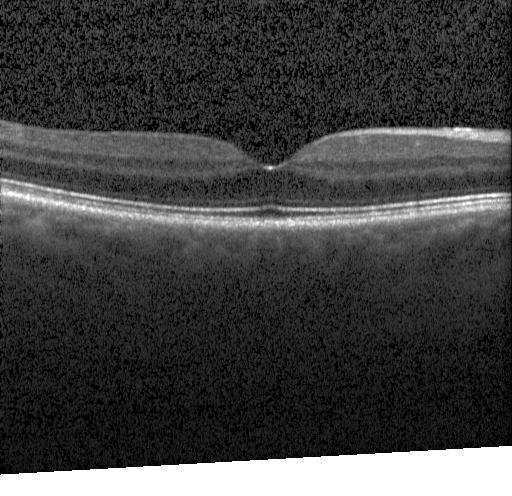 Centered on the fovea. SD-OCT. OCT B-scan
Finding: no choroidal neovascularization, diabetic macular edema, or drusen.